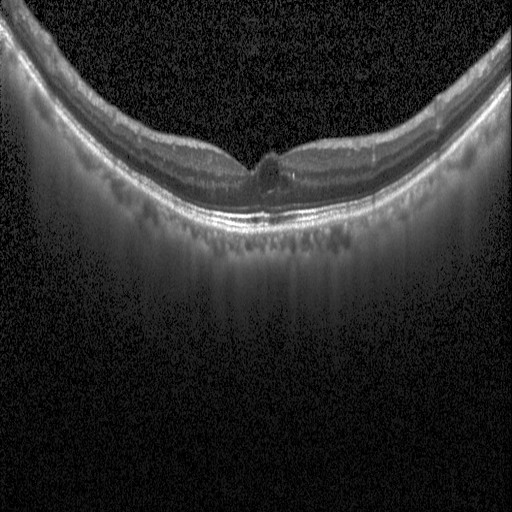 Retinal OCT cross-section showing diabetic macular edema.